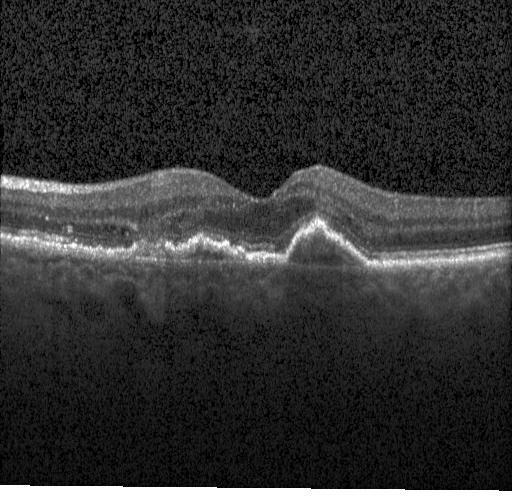 Centered on the fovea; spectral-domain optical coherence tomography; instrument: Heidelberg Spectralis; optical coherence tomography B-scan
Finding: a choroidal neovascular membrane.